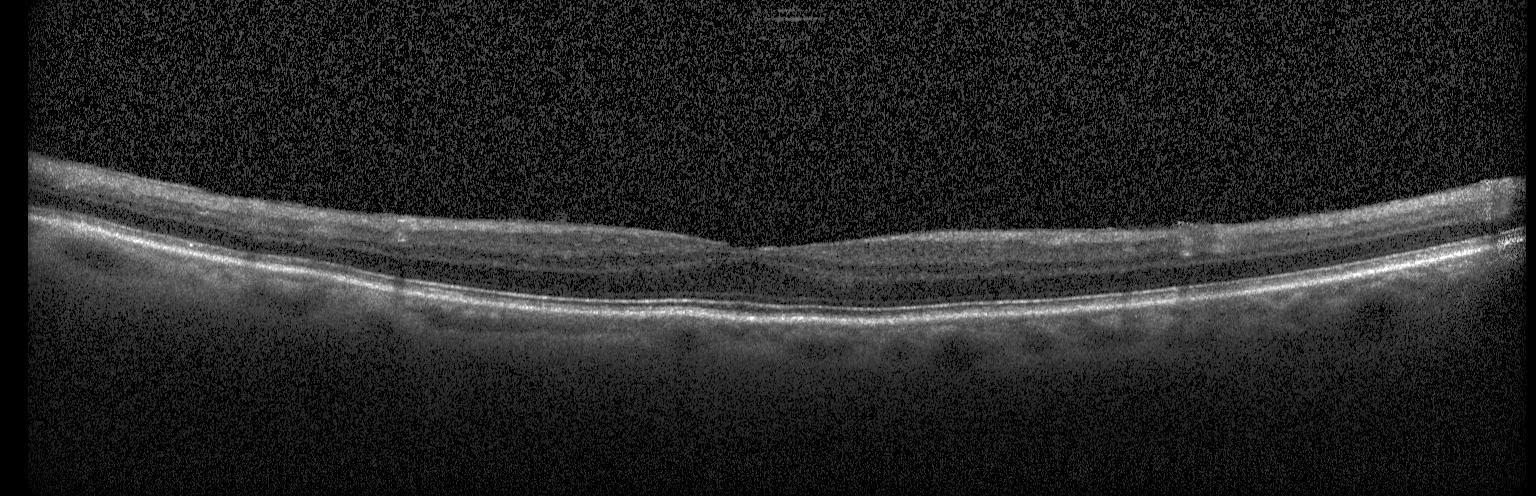
OCT line scan · fovea-centered.
The scan shows no choroidal neovascularization, no diabetic macular edema, and no drusen.